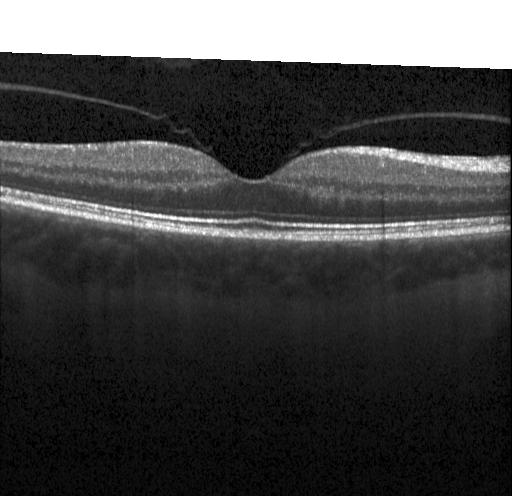

This B-scan demonstrates no choroidal neovascularization, diabetic macular edema, or drusen.